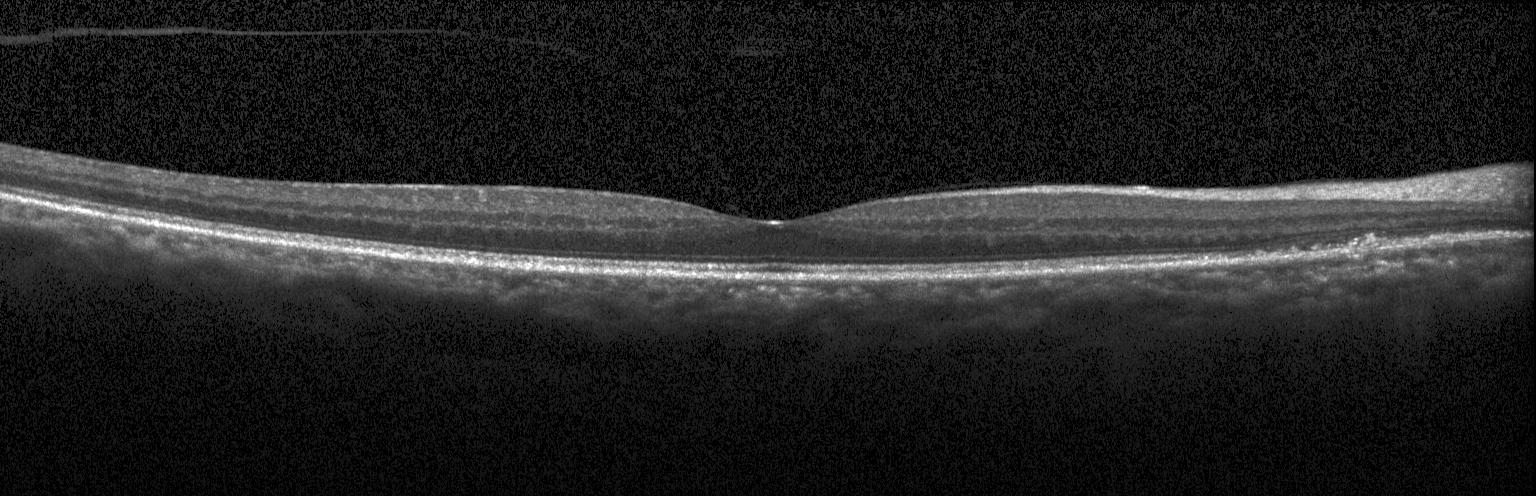
The scan shows no choroidal neovascularization, diabetic macular edema, or drusen.